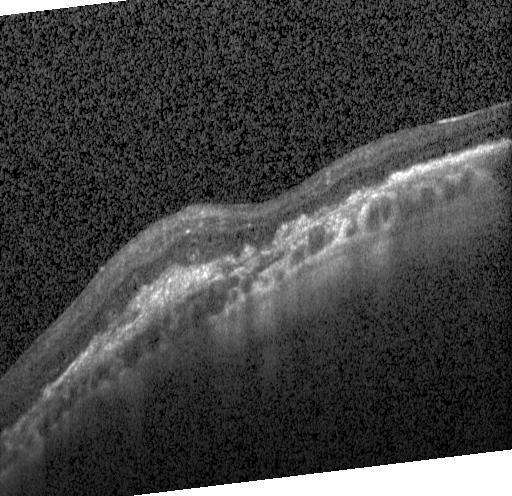 OCT scan showing a choroidal neovascular membrane.